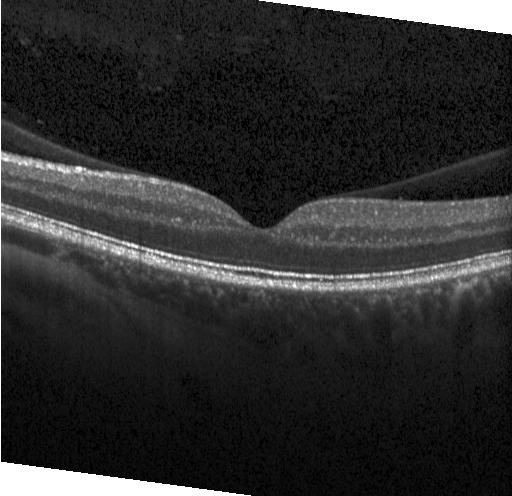
Retinal OCT B-scan. Dx: no evidence of choroidal neovascularization, diabetic macular edema, or drusen.